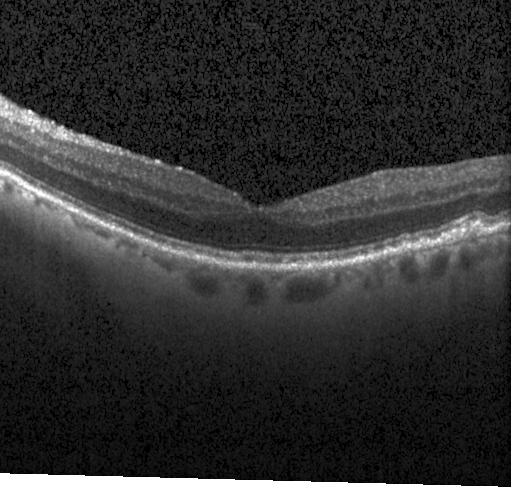

Spectral-domain OCT · OCT line scan · through the macula
Multiple drusen.